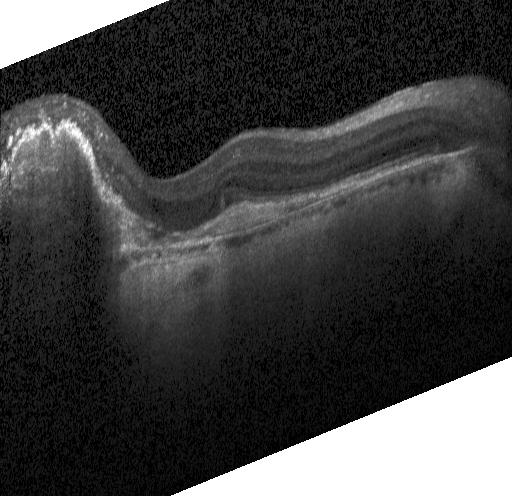

Finding: a choroidal neovascular membrane.